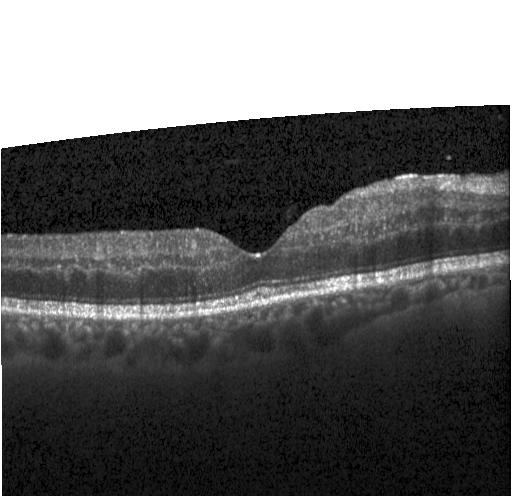 OCT finding: no choroidal neovascularization, diabetic macular edema, or drusen.